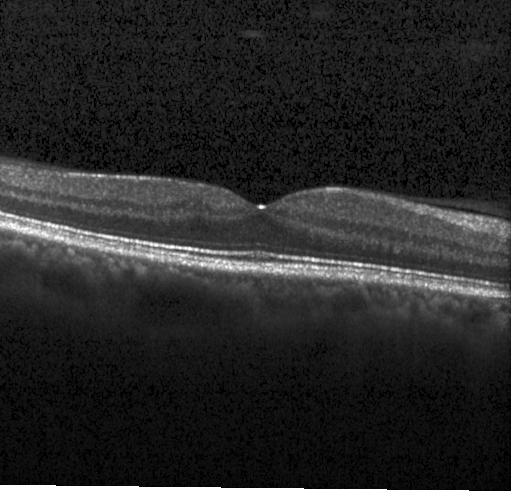 Horizontal scan through the fovea; spectral-domain optical coherence tomography; OCT line scan; Heidelberg Spectralis OCT system
The scan shows neither choroidal neovascularization, diabetic macular edema, nor drusen.